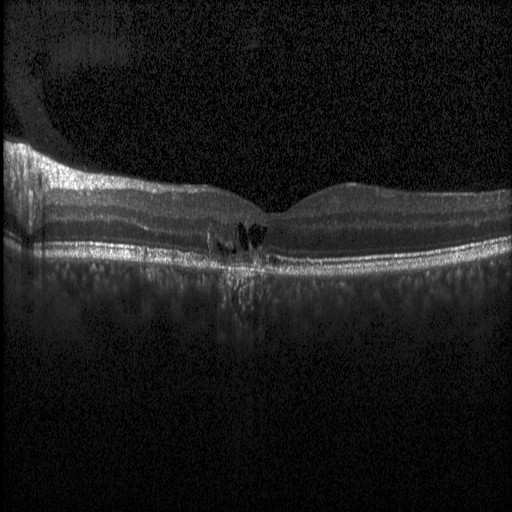

Horizontal scan through the fovea, instrument: Heidelberg Spectralis, OCT line scan, spectral-domain optical coherence tomography.
Diabetic macular edema (DME).